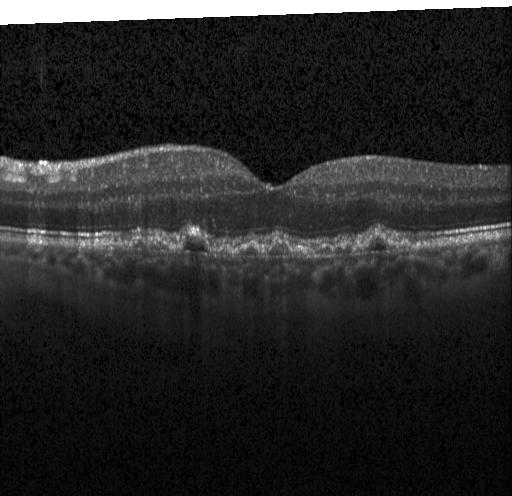
Macular OCT demonstrating drusen.